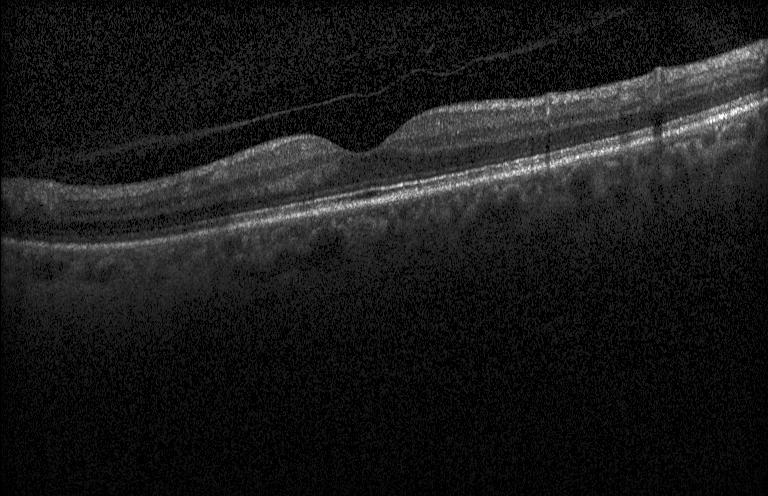
OCT B-scan — Neither choroidal neovascularization, diabetic macular edema, nor drusen.